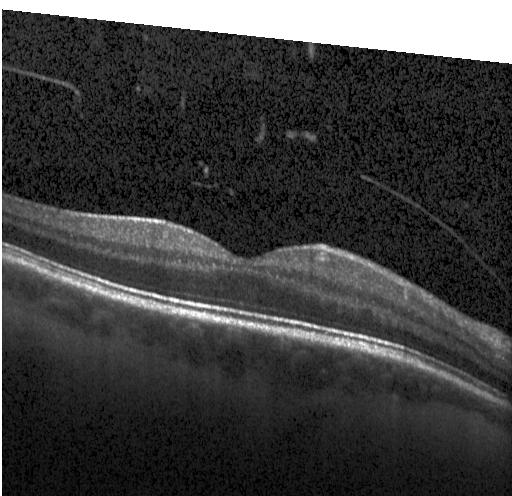

OCT line scan. This B-scan demonstrates no choroidal neovascularization, no diabetic macular edema, and no drusen.